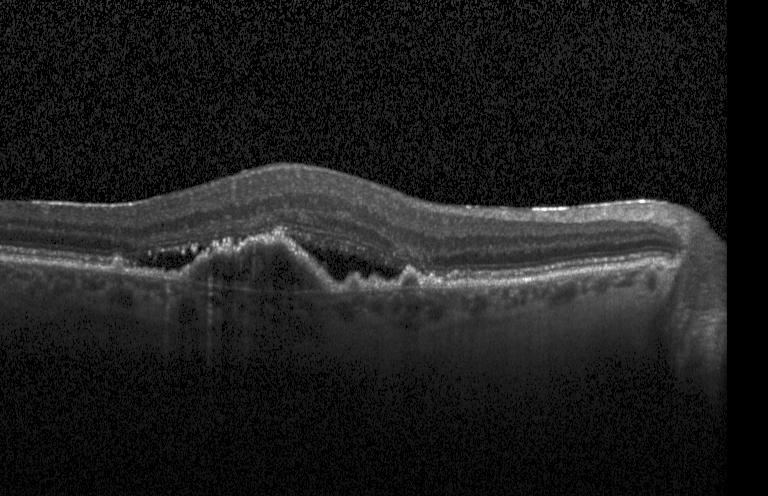
OCT line scan, acquired on a Heidelberg Spectralis.
Impression: a choroidal neovascular membrane.